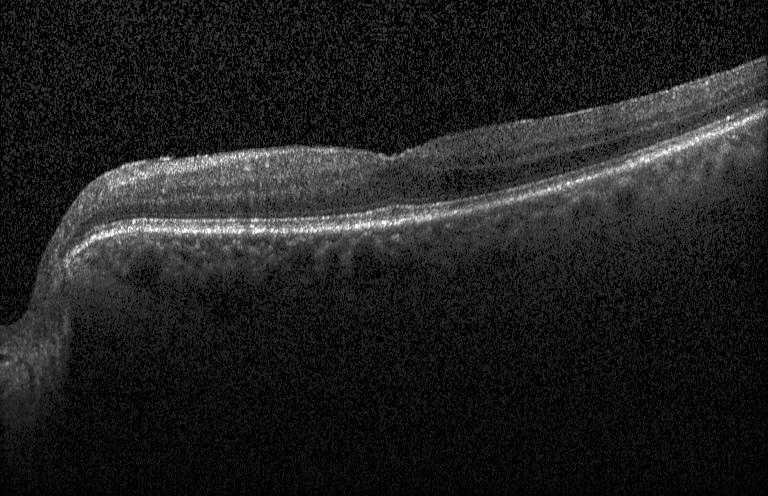

Acquired on a Heidelberg Spectralis, retinal OCT B-scan, SD-OCT, macular scan.
Finding: neither CNV, DME, nor drusen.